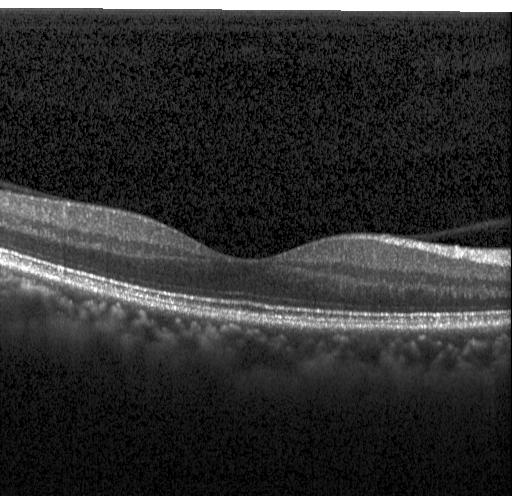
OCT line scan · fovea-centered · spectral-domain OCT · Heidelberg Spectralis. Diagnosis: no CNV, no DME, and no drusen.